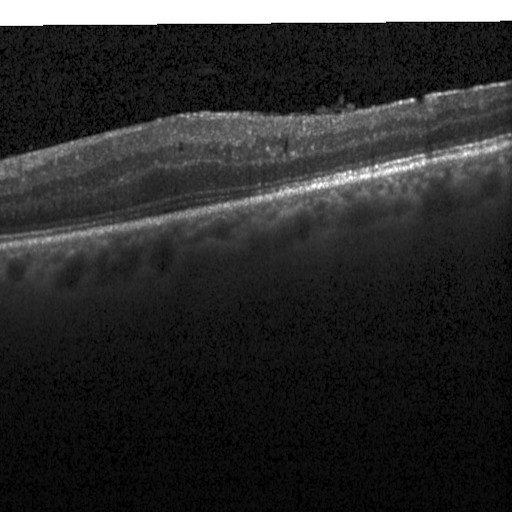

Retinal OCT B-scan
Dx: DME.